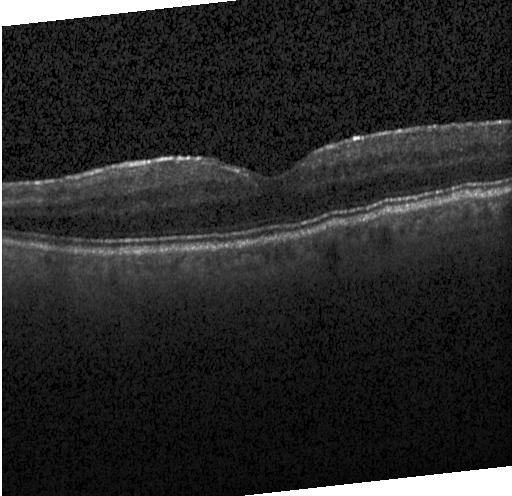
Impression: no choroidal neovascularization, diabetic macular edema, or drusen.